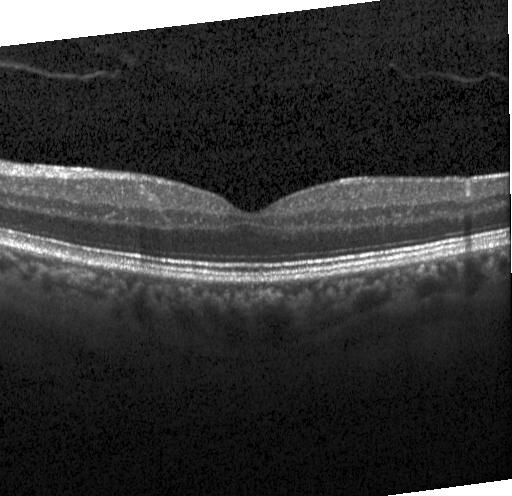
Horizontal scan through the fovea, optical coherence tomography scan, instrument: Heidelberg Spectralis.
Diagnosis: no CNV, no DME, and no drusen.